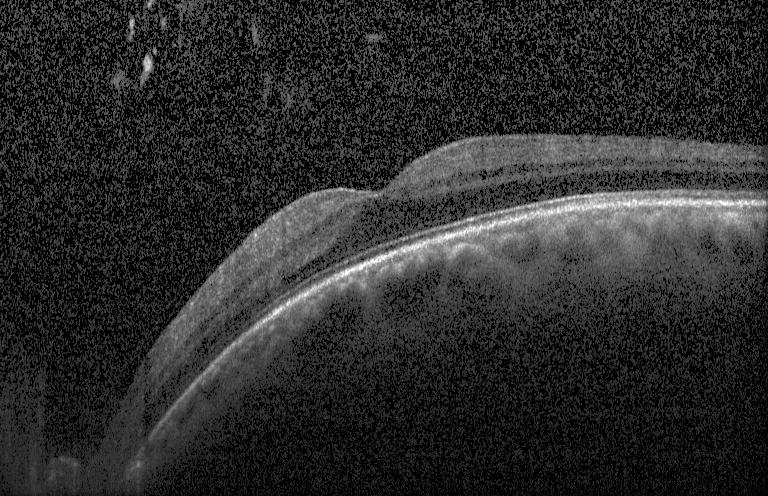

Acquired on a Heidelberg Spectralis, centered on the fovea, spectral-domain optical coherence tomography, optical coherence tomography B-scan. This B-scan demonstrates no choroidal neovascularization, diabetic macular edema, or drusen.